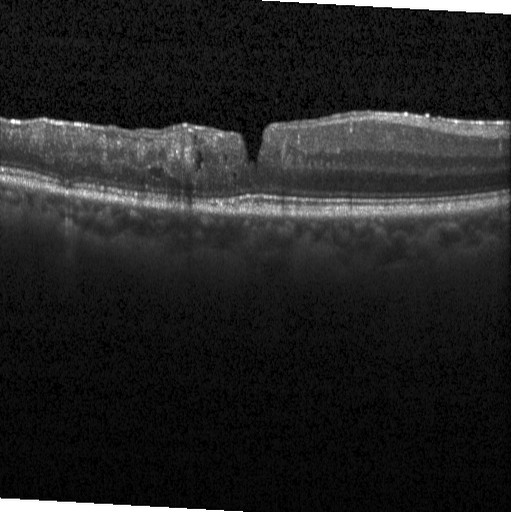

OCT finding: diabetic macular edema (DME).